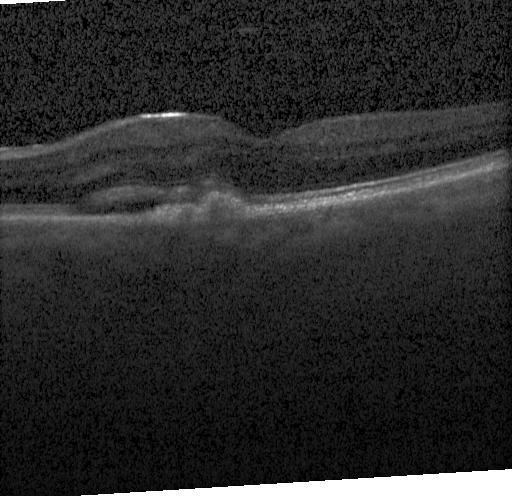
The scan shows choroidal neovascularization.